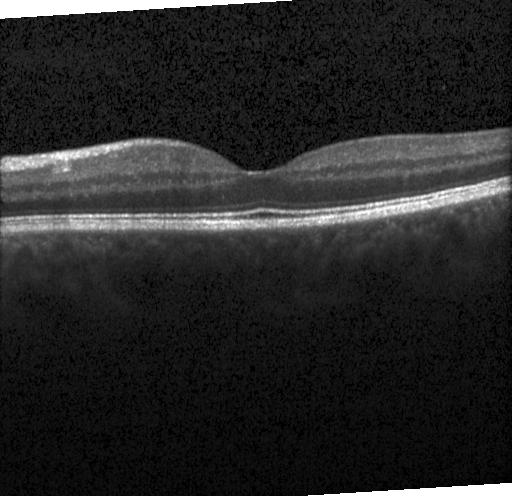 Macular OCT demonstrating no CNV, no DME, and no drusen.